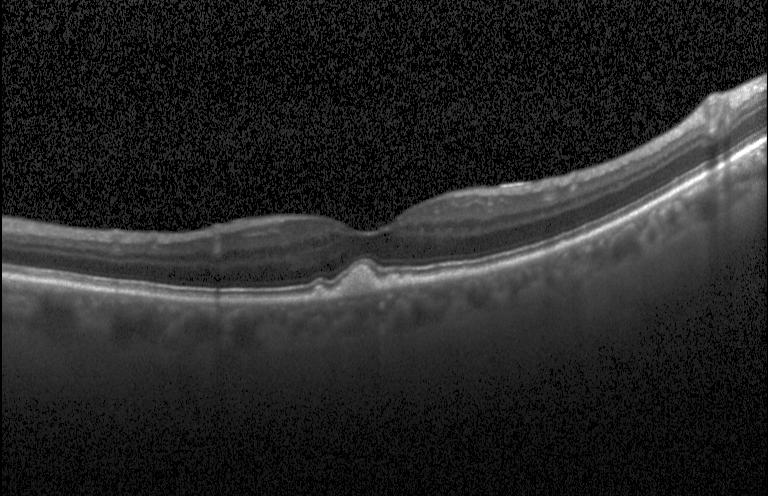 SD-OCT; centered on the fovea; optical coherence tomography B-scan.
Diagnosis: sub-RPE drusenoid deposits.